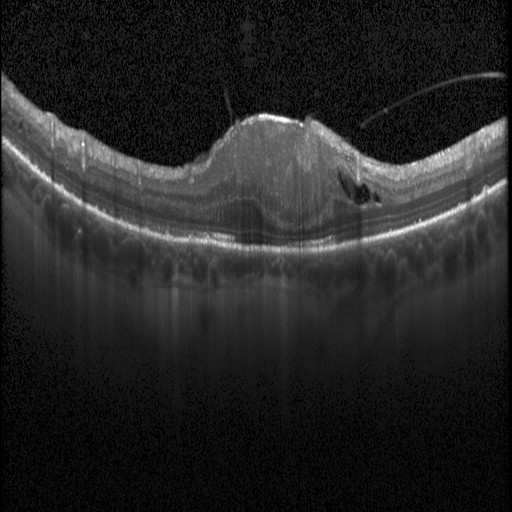
OCT finding: diabetic macular edema.